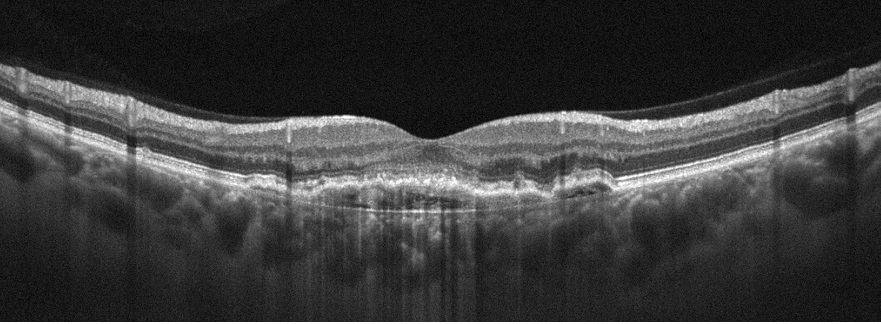 Through the macula, OCT B-scan.
Dx: age-related macular degeneration (AMD).